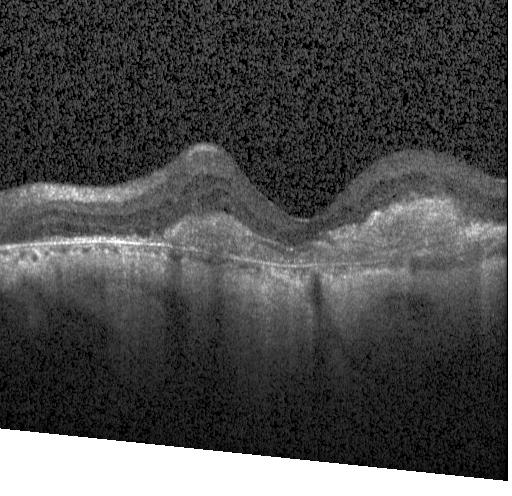
Centered on the fovea. Spectral-domain optical coherence tomography. Retinal OCT B-scan.
Assessment: a choroidal neovascular membrane.